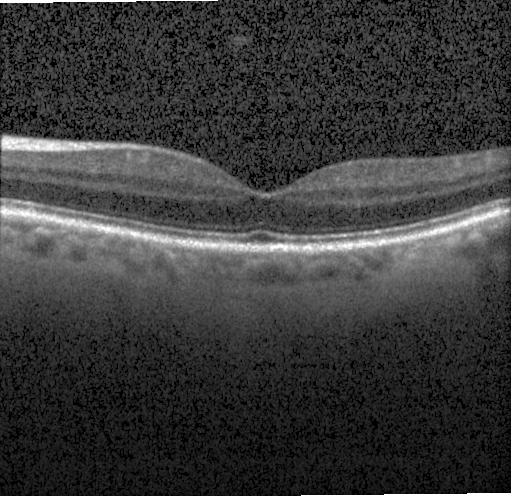

OCT line scan; macular scan.
Neither choroidal neovascularization, diabetic macular edema, nor drusen.